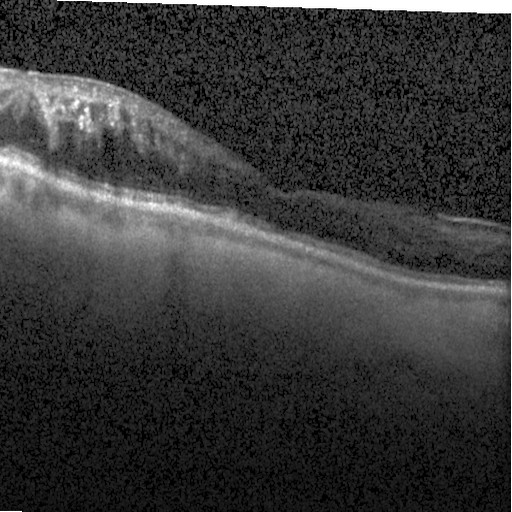
Finding: DME.